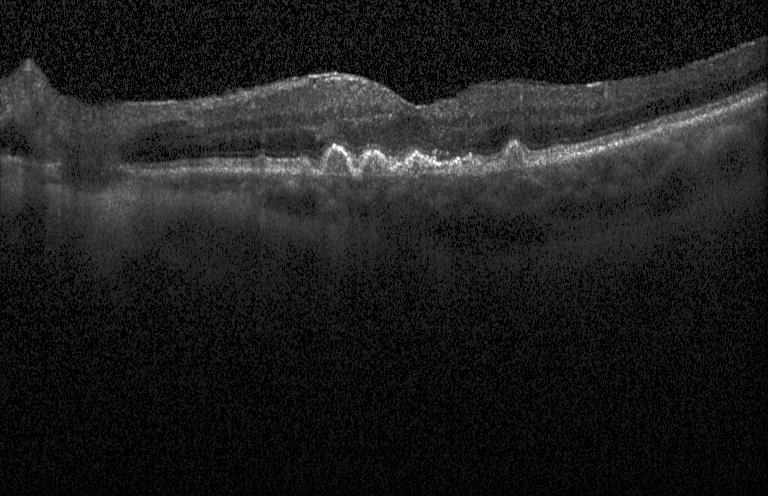 Macular OCT: sub-RPE drusenoid deposits.